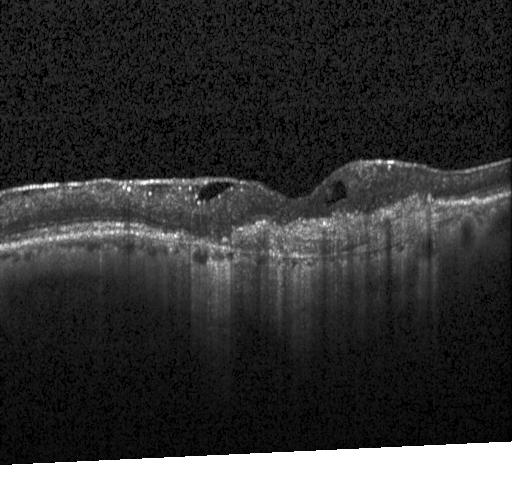
Spectral-domain OCT · instrument: Heidelberg Spectralis · through the macula · retinal OCT B-scan.
Macular OCT: choroidal neovascularization (CNV).